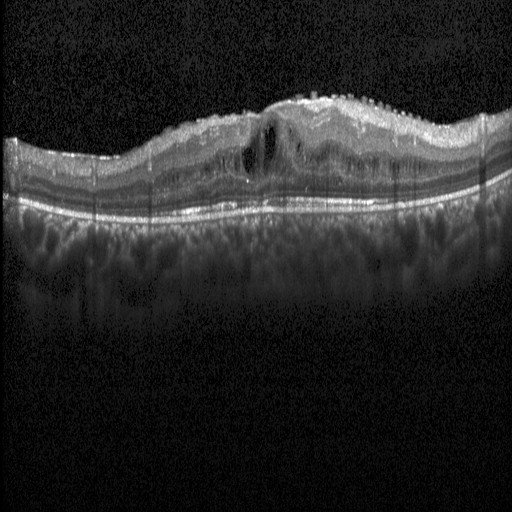

OCT line scan — Impression: diabetic macular edema.